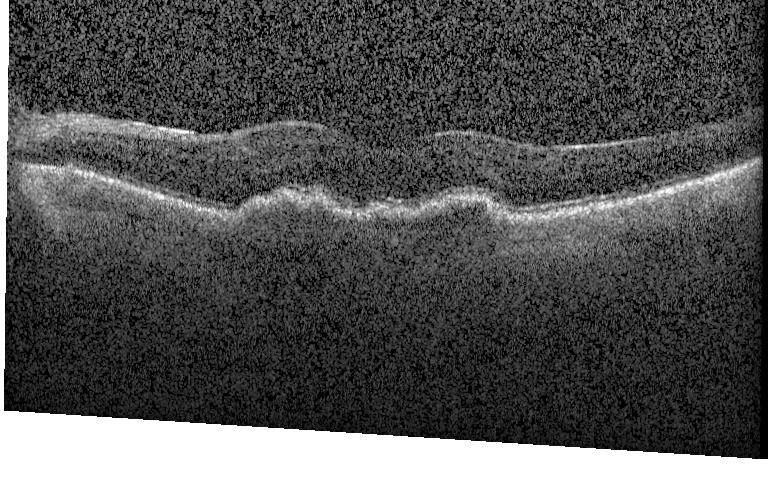

Fovea-centered, retinal OCT B-scan.
Finding: a choroidal neovascular membrane.